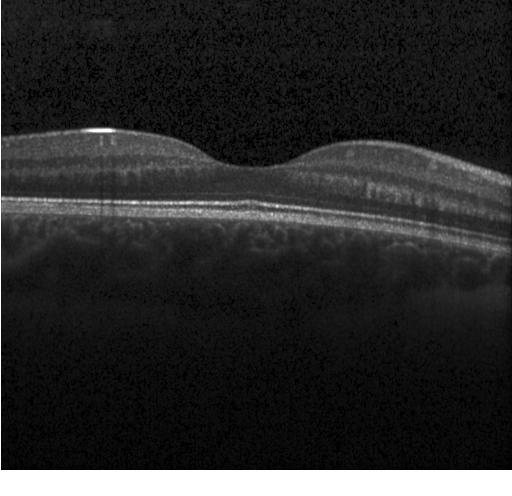
Spectral-domain optical coherence tomography · optical coherence tomography B-scan · acquired on a Heidelberg Spectralis · fovea-centered.
Impression: no choroidal neovascularization, diabetic macular edema, or drusen.